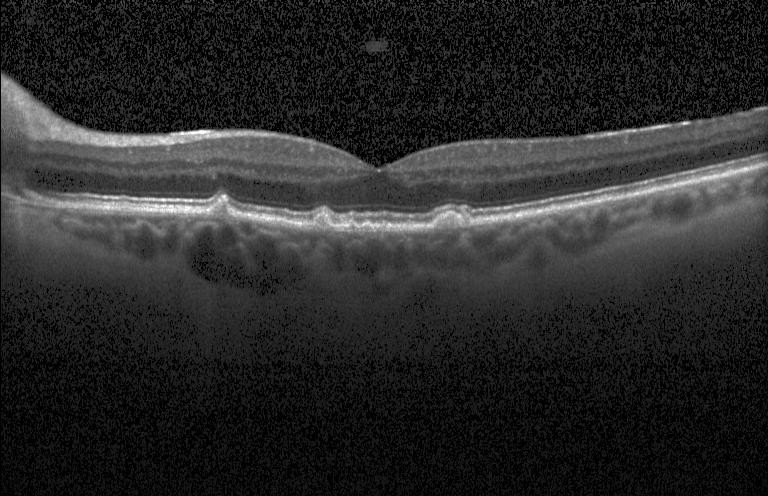

This B-scan demonstrates multiple drusen.